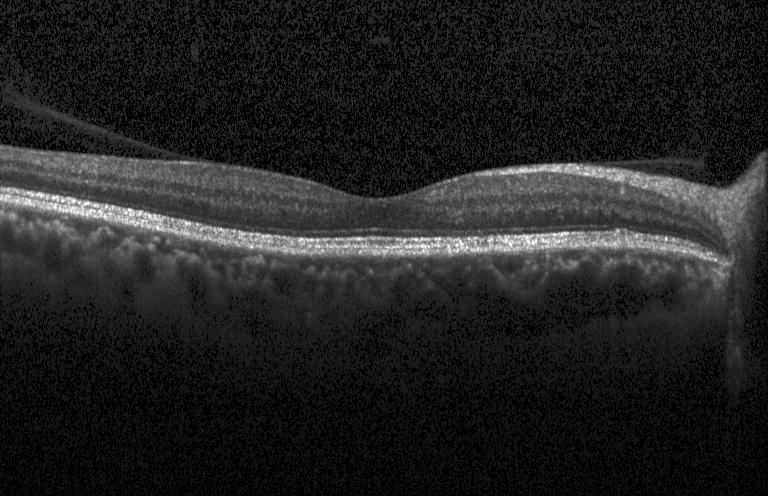 Optical coherence tomography B-scan. Heidelberg Spectralis.
Dx: neither choroidal neovascularization, diabetic macular edema, nor drusen.